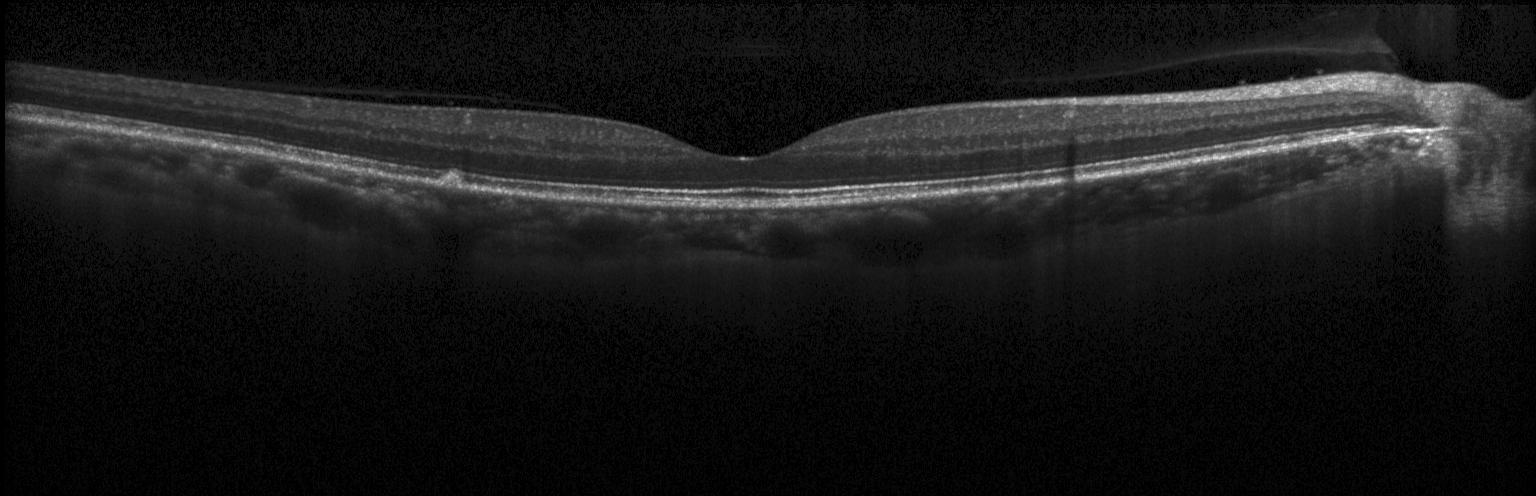
Optical coherence tomography B-scan. Spectral-domain optical coherence tomography. This B-scan demonstrates multiple drusen.